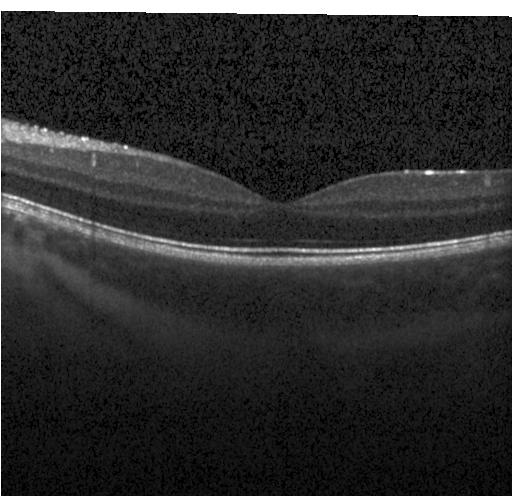

OCT line scan; instrument: Heidelberg Spectralis; spectral-domain OCT; macular scan. No evidence of choroidal neovascularization, diabetic macular edema, or drusen.